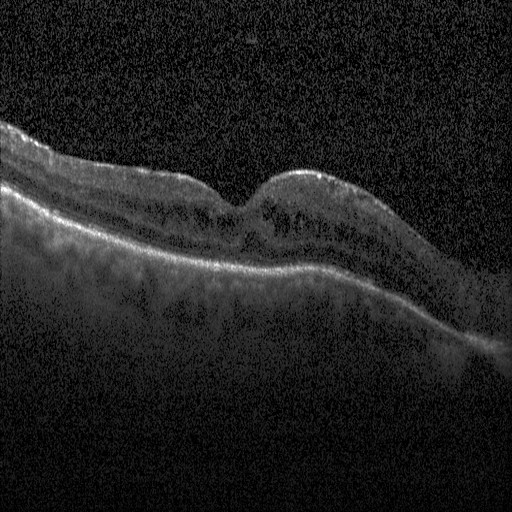
Dx: diabetic macular edema.